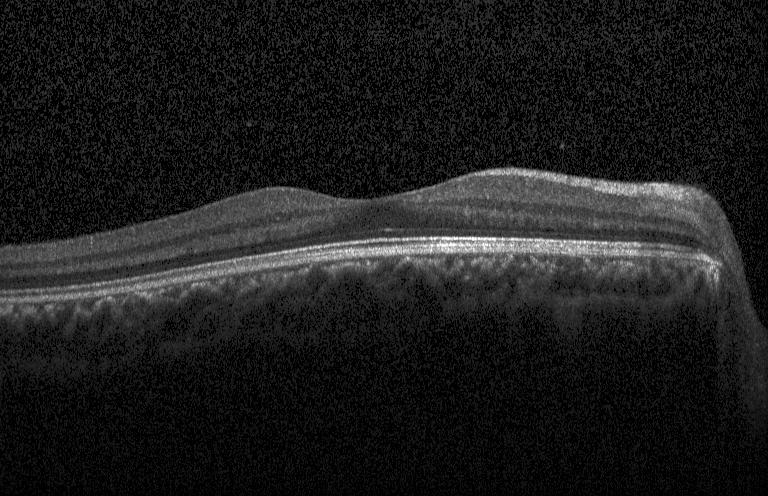
Horizontal scan through the fovea. Retinal OCT cross-section. Spectral-domain optical coherence tomography. Heidelberg Spectralis OCT system
Assessment: no choroidal neovascularization, diabetic macular edema, or drusen.